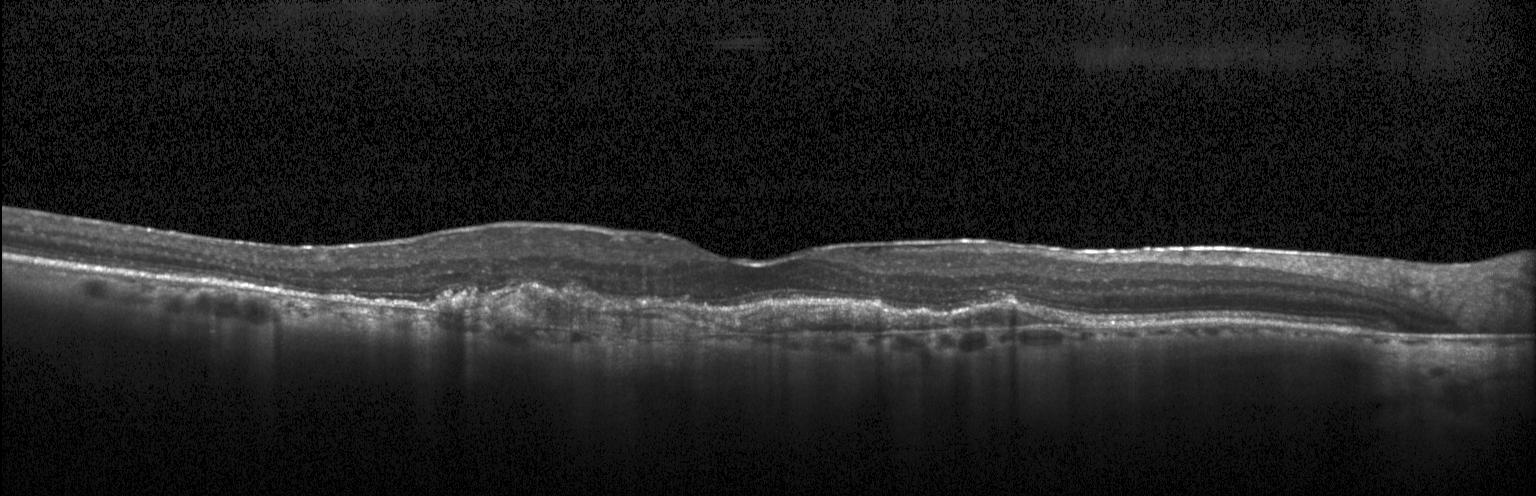

OCT B-scan showing CNV.